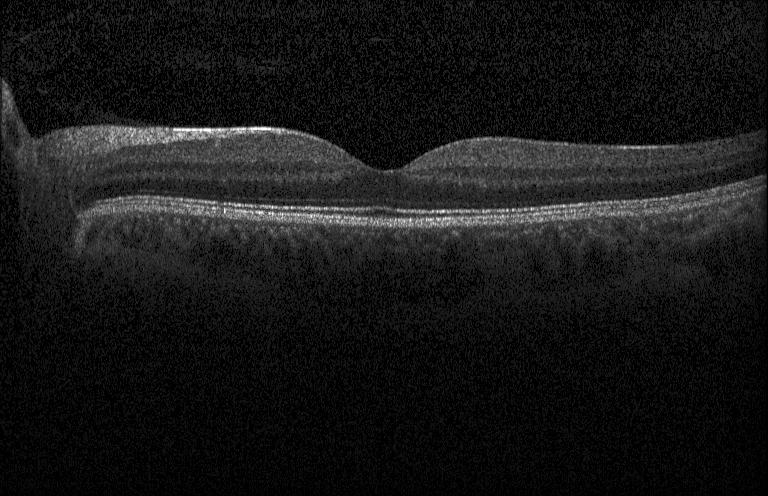 OCT B-scan.
Dx: no choroidal neovascularization, no diabetic macular edema, and no drusen.